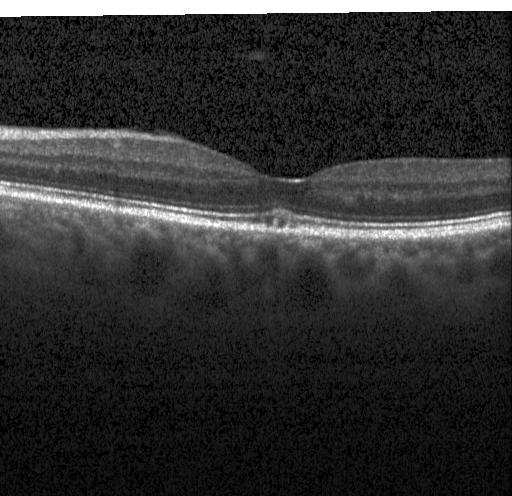

Retinal OCT B-scan — Finding: no choroidal neovascularization, no diabetic macular edema, and no drusen.